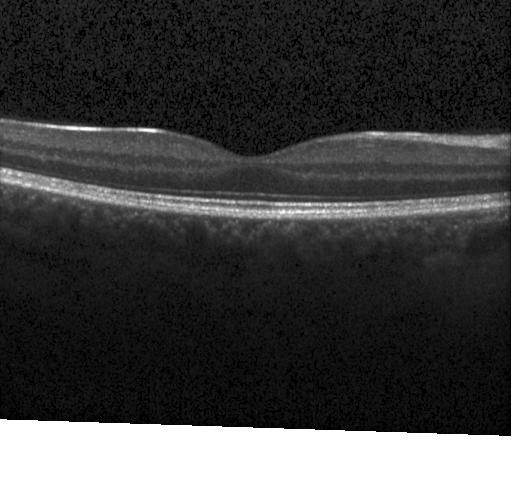 OCT B-scan
Finding: no evidence of CNV, DME, or drusen.